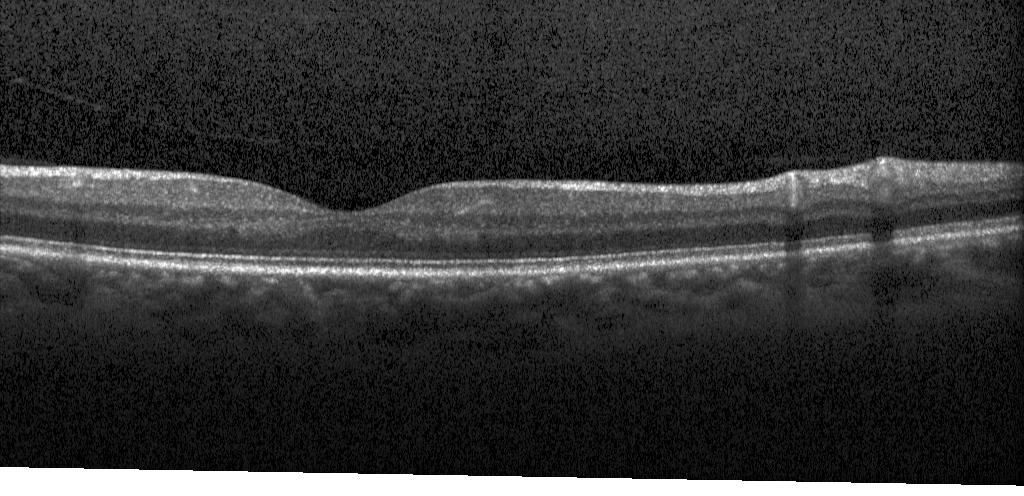
Retinal OCT B-scan.
No choroidal neovascularization, no diabetic macular edema, and no drusen.